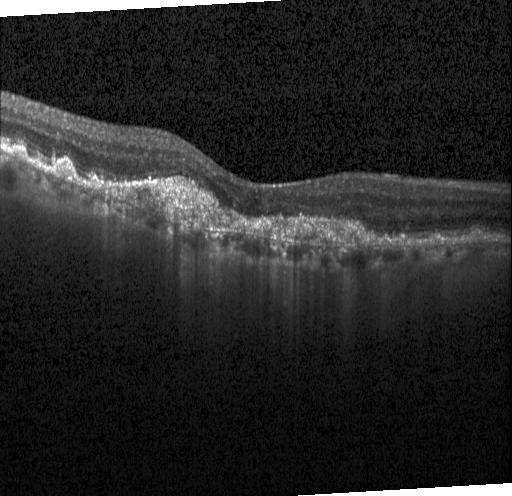 Diagnosis: CNV.